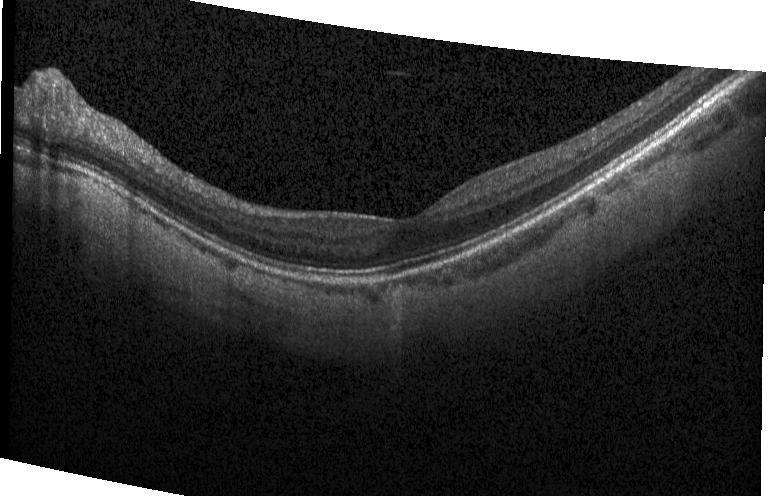 Retinal OCT B-scan, spectral-domain OCT
Finding: no choroidal neovascularization, no diabetic macular edema, and no drusen.